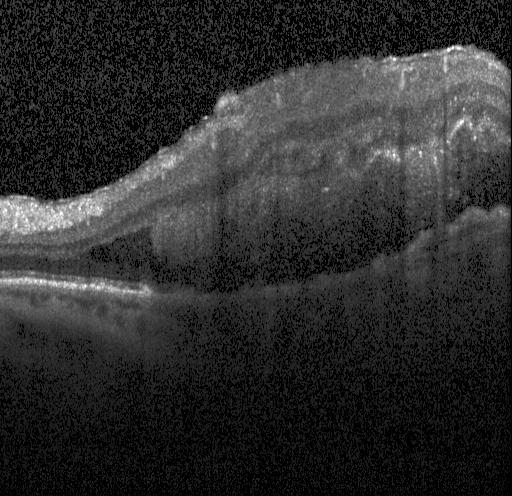

Impression: choroidal neovascularization (CNV).